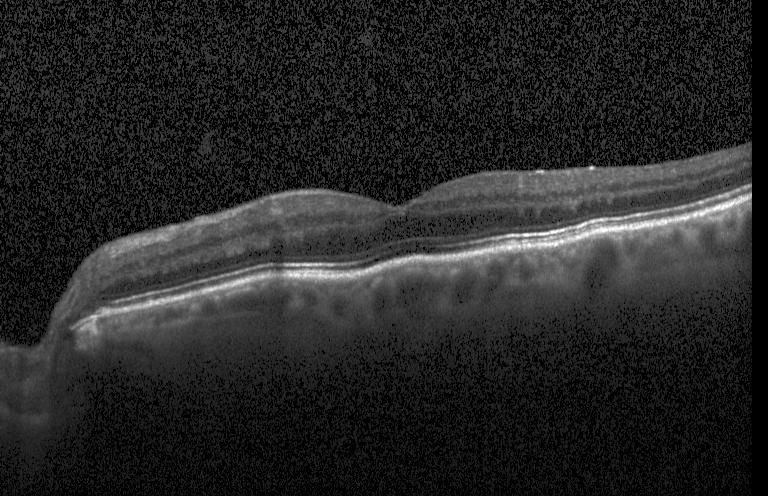 Retinal OCT B-scan. Spectral-domain optical coherence tomography — Macular OCT: no evidence of CNV, DME, or drusen.